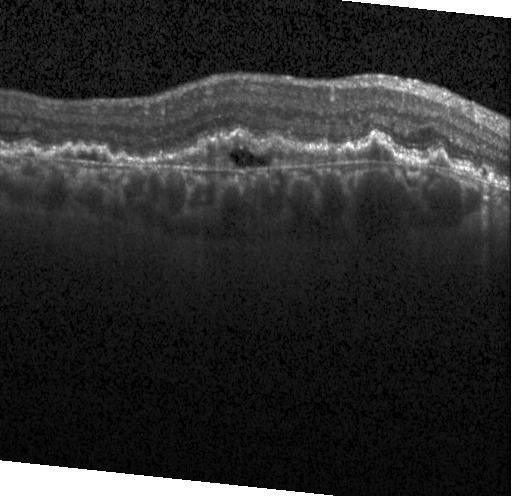
This B-scan demonstrates choroidal neovascularization.